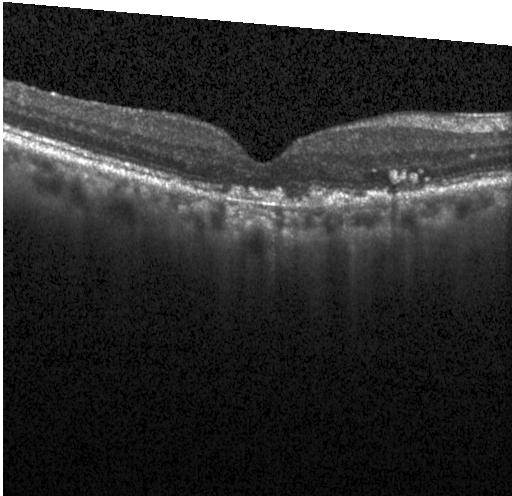 Fovea-centered, instrument: Heidelberg Spectralis, retinal OCT cross-section. OCT finding: a choroidal neovascular membrane.